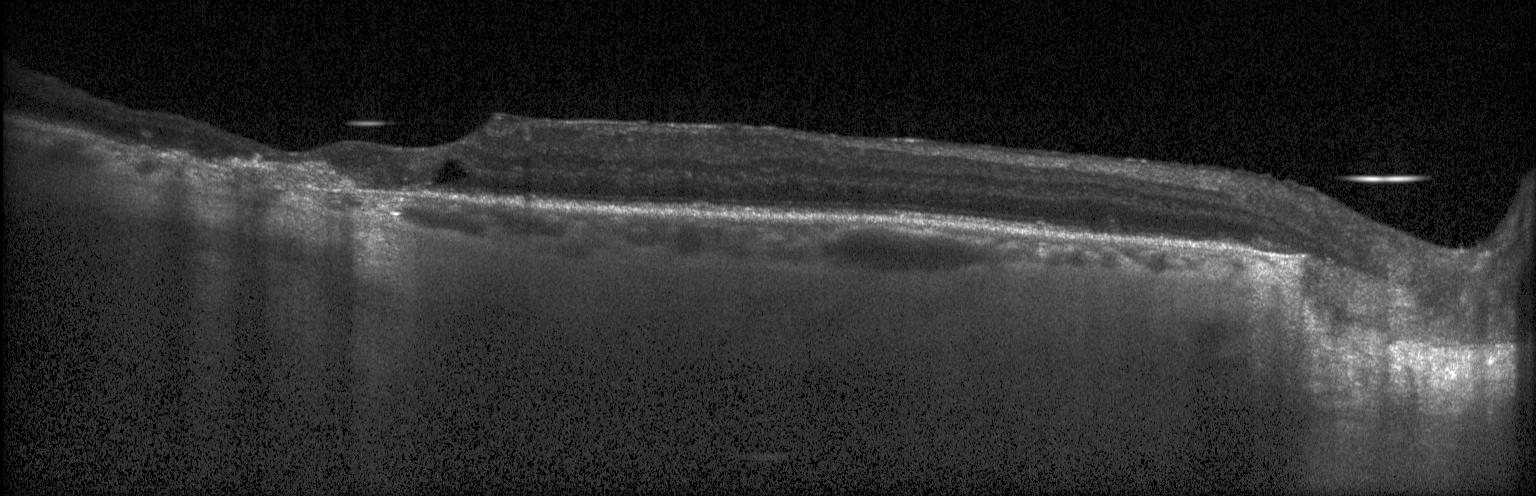 Instrument: Heidelberg Spectralis; spectral-domain OCT; horizontal scan through the fovea; retinal OCT cross-section. Diagnosis: choroidal neovascularization.